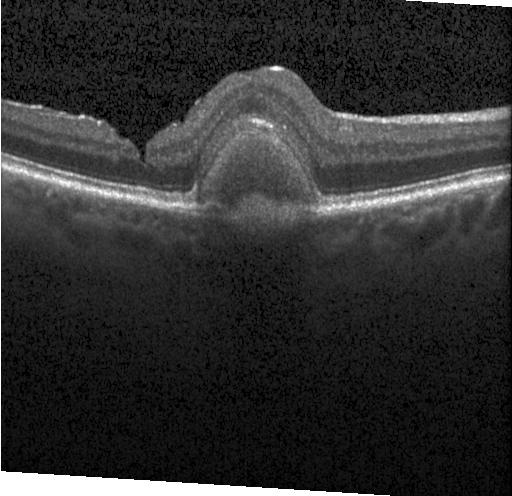
Optical coherence tomography scan — Assessment: CNV.